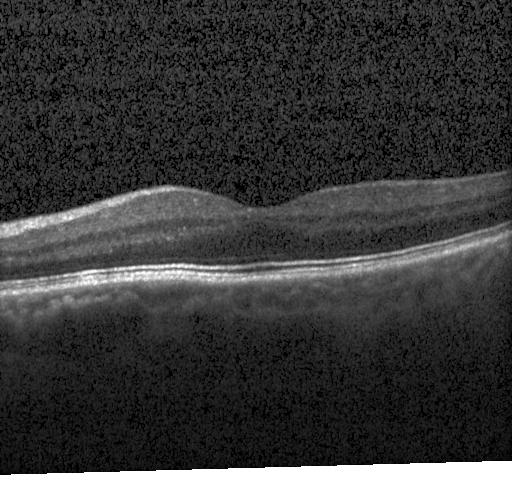 Diagnosis: no choroidal neovascularization, no diabetic macular edema, and no drusen.